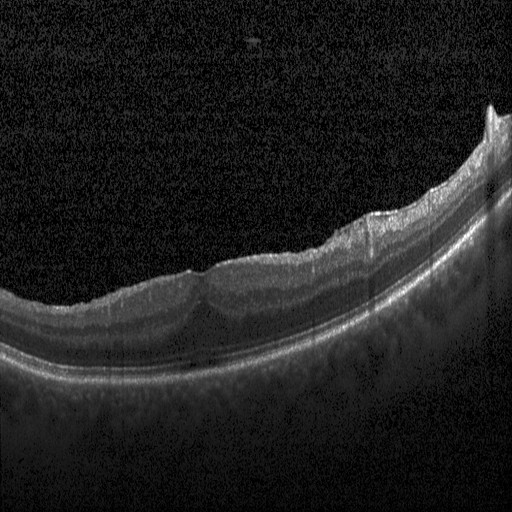 Optical coherence tomography B-scan — This B-scan demonstrates diabetic macular edema (DME).